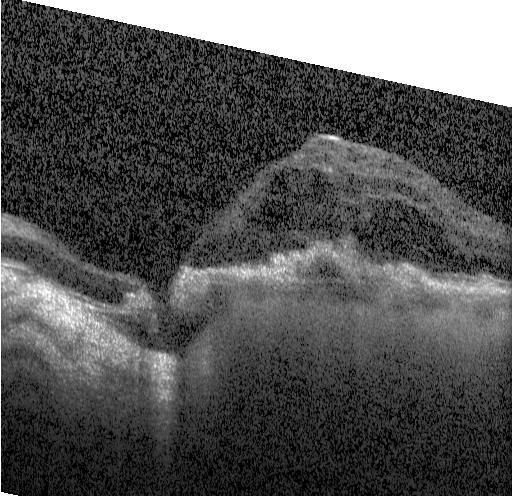

Finding: choroidal neovascularization (CNV).